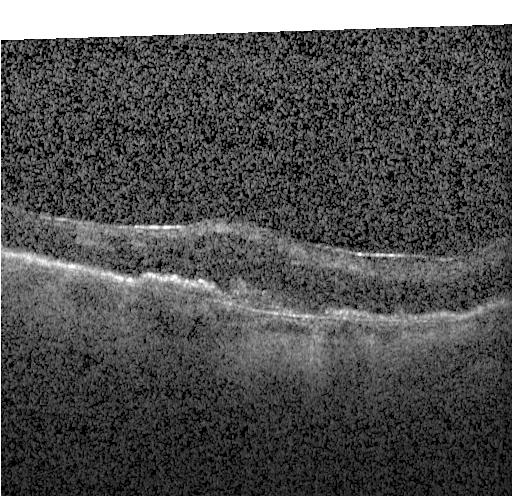 Diagnosis: a choroidal neovascular membrane.